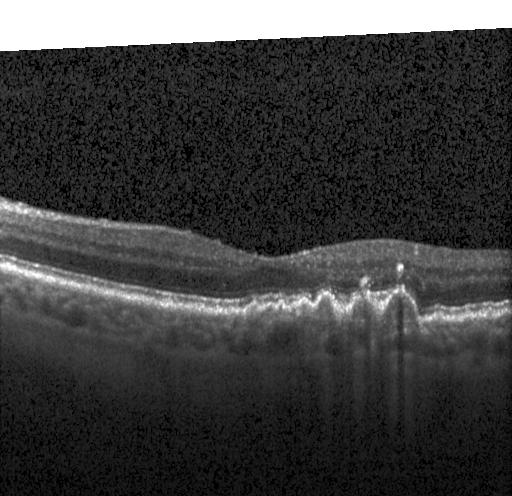
Heidelberg Spectralis OCT system, OCT B-scan
Finding: multiple drusen.